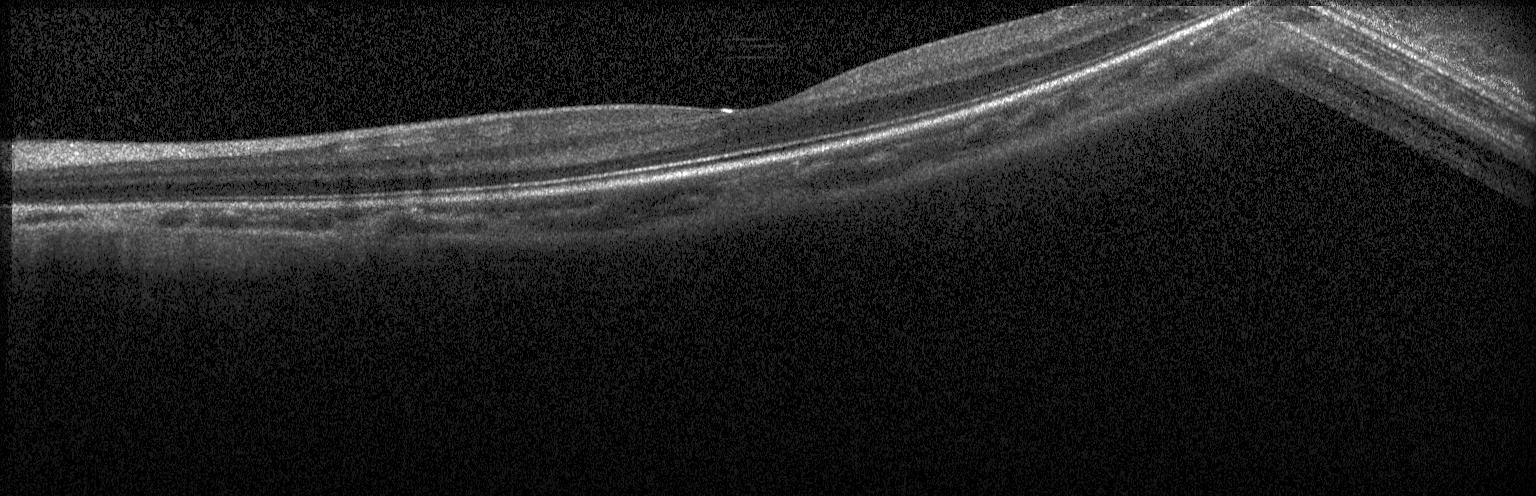
Finding: no evidence of choroidal neovascularization, diabetic macular edema, or drusen.